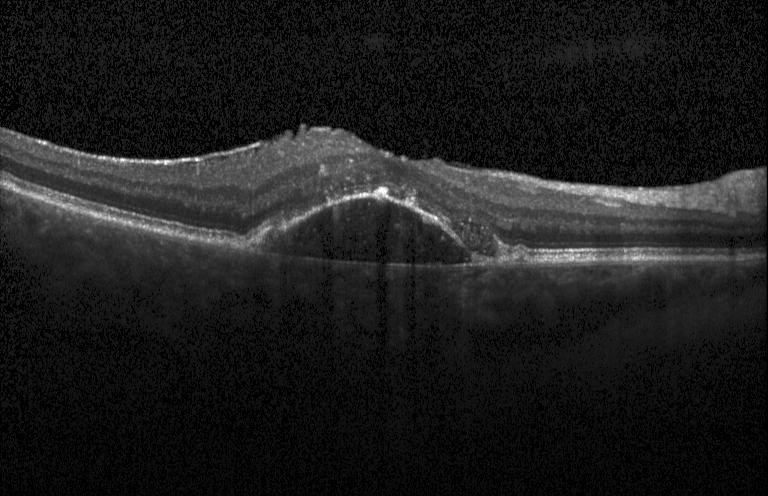 Optical coherence tomography scan; instrument: Heidelberg Spectralis
This B-scan demonstrates a choroidal neovascular membrane.